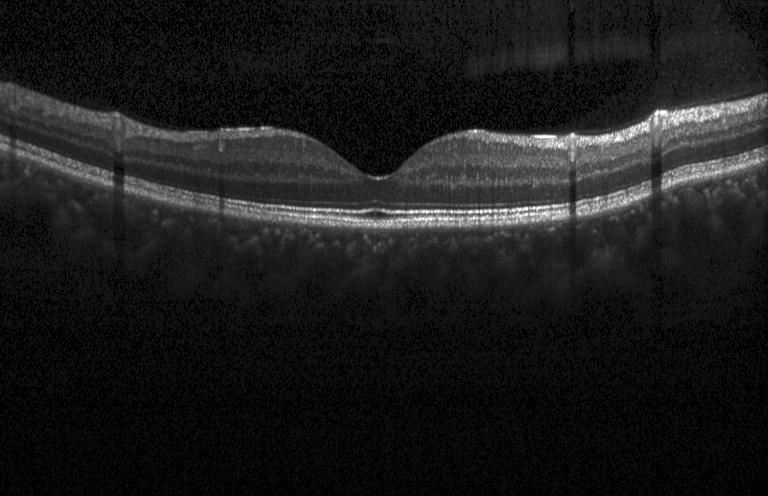
Retinal OCT B-scan.
Dx: no choroidal neovascularization, no diabetic macular edema, and no drusen.